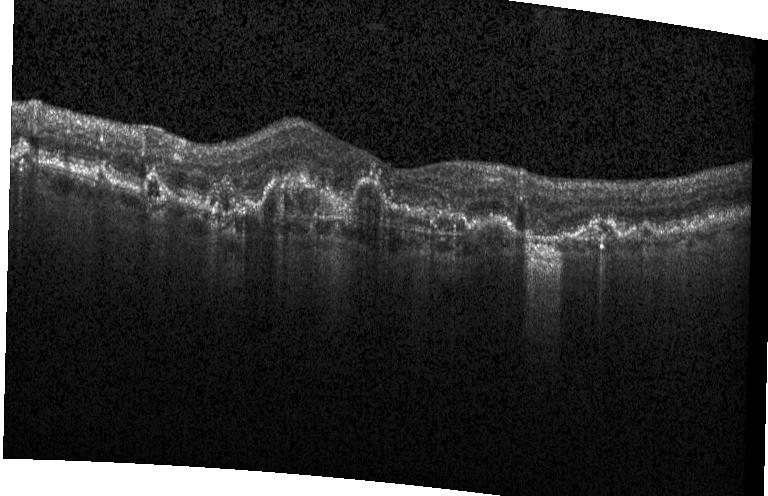 Retinal OCT cross-section showing CNV.